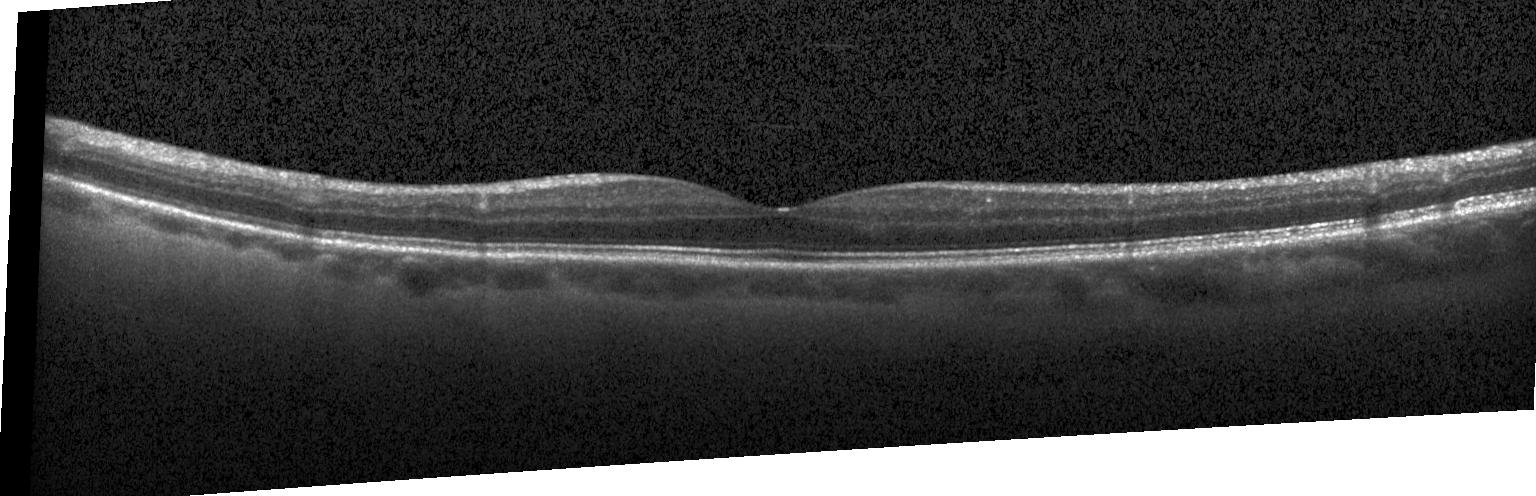 Impression: no choroidal neovascularization, no diabetic macular edema, and no drusen.